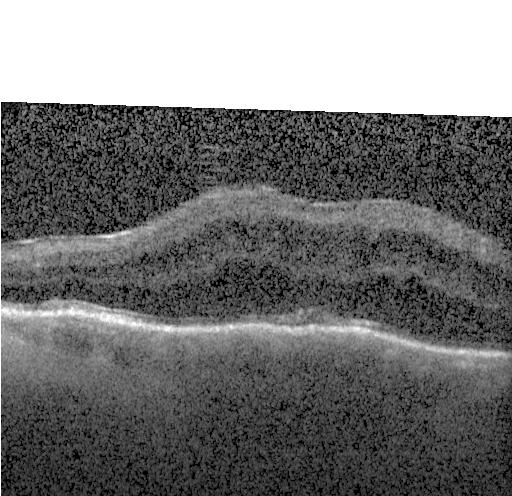 Optical coherence tomography B-scan; centered on the fovea; instrument: Heidelberg Spectralis; spectral-domain OCT
Assessment: DME.